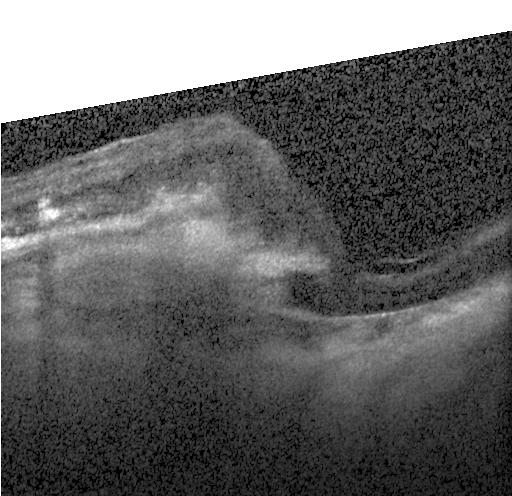 Retinal OCT B-scan — Finding: a choroidal neovascular membrane.